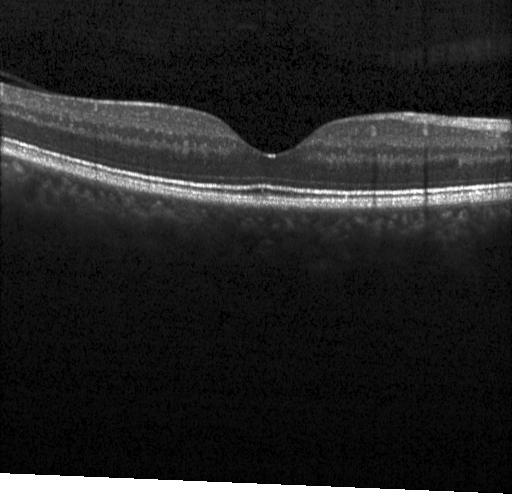 OCT B-scan — Diagnosis: no CNV, DME, or drusen.